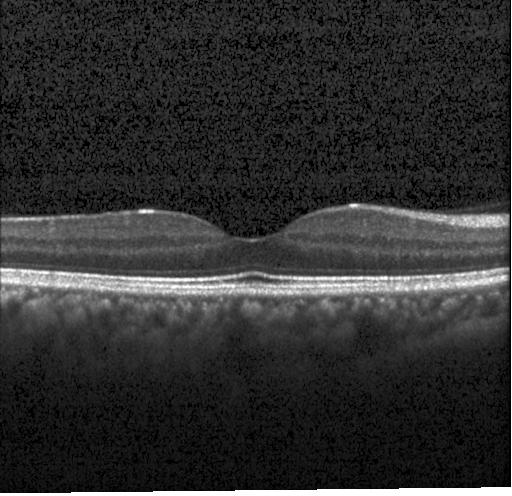 Heidelberg Spectralis; OCT line scan.
Diagnosis: no evidence of choroidal neovascularization, diabetic macular edema, or drusen.